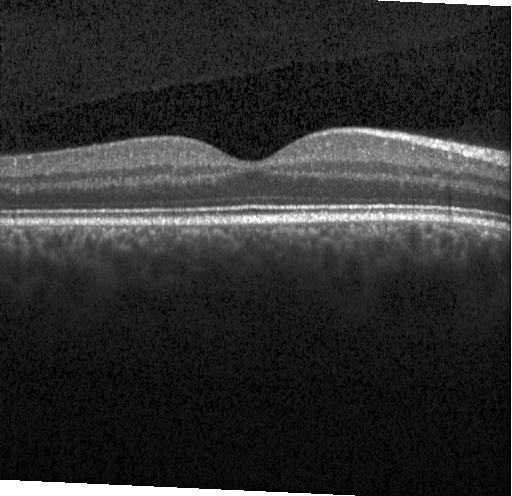 Optical coherence tomography scan · spectral-domain optical coherence tomography · instrument: Heidelberg Spectralis.
This B-scan demonstrates no evidence of choroidal neovascularization, diabetic macular edema, or drusen.